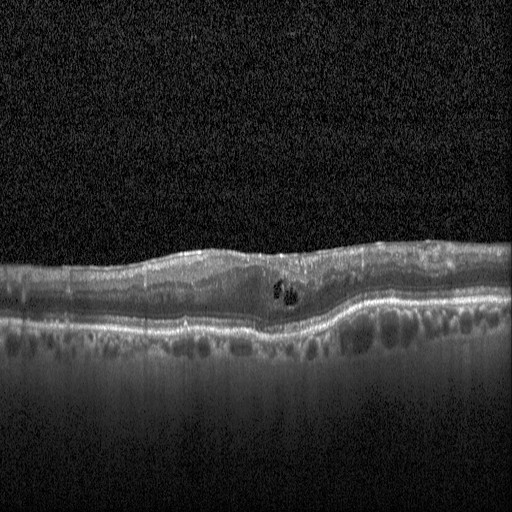
Diagnosis: diabetic macular edema.